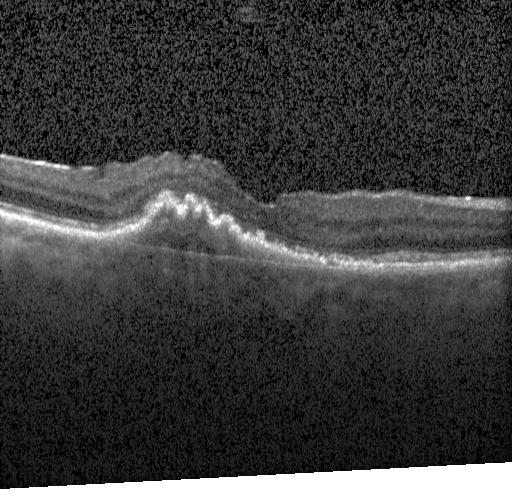 OCT scan showing a choroidal neovascular membrane.